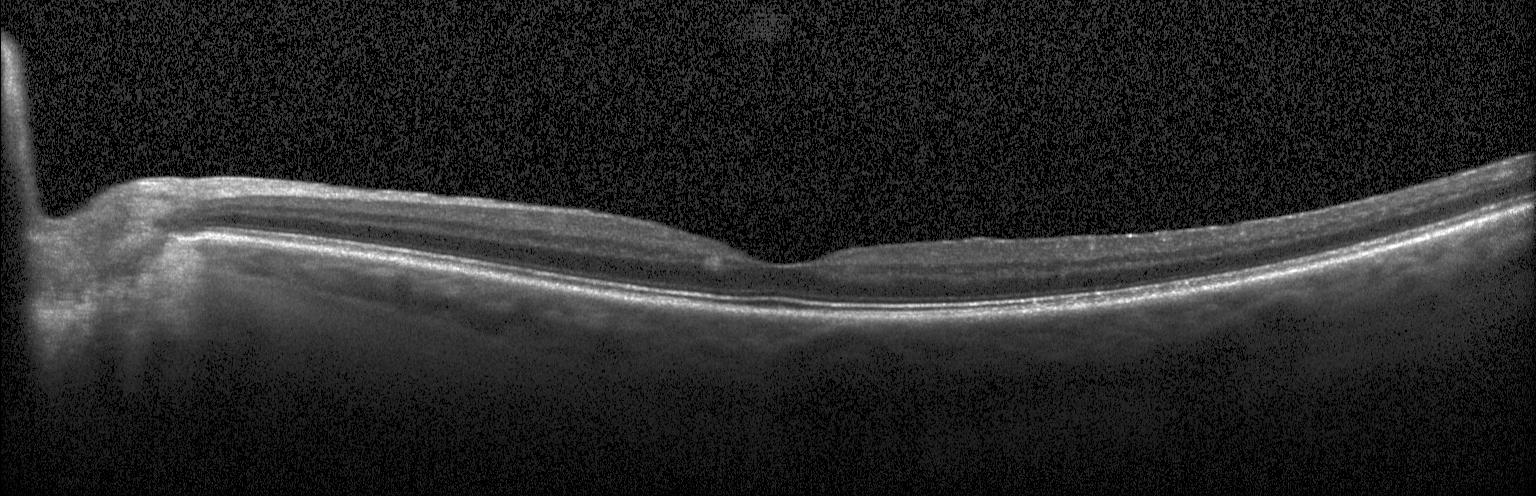 OCT B-scan showing neither choroidal neovascularization, diabetic macular edema, nor drusen.